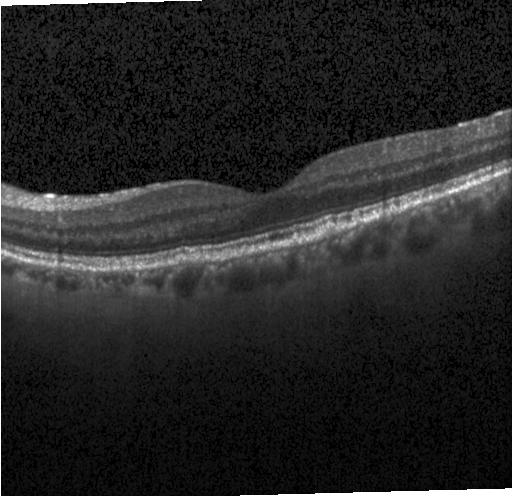

Spectral-domain OCT B-scan: multiple drusen.